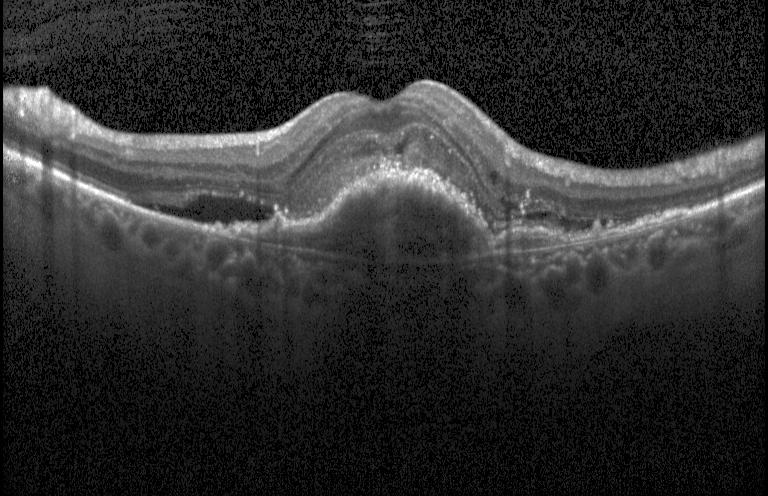 OCT B-scan showing CNV.